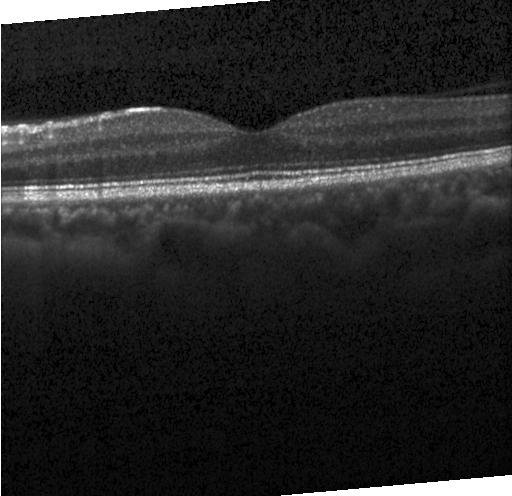 Macular OCT: no CNV, no DME, and no drusen.